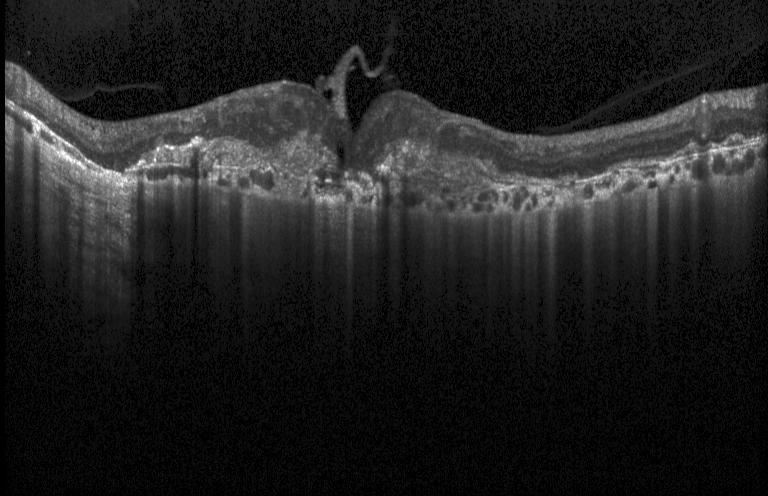 Instrument: Heidelberg Spectralis; optical coherence tomography scan; SD-OCT; fovea-centered
Finding: a choroidal neovascular membrane.